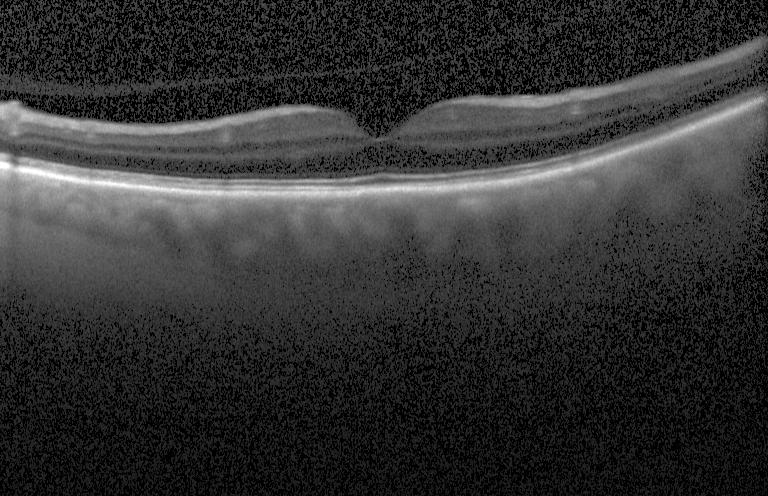 Centered on the fovea · retinal OCT B-scan.
Dx: no choroidal neovascularization, diabetic macular edema, or drusen.